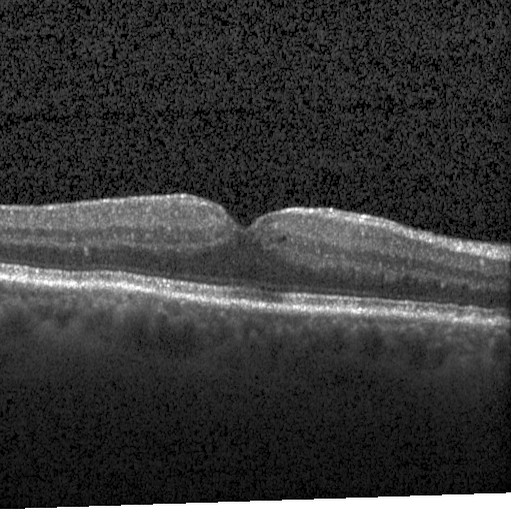

Impression: DME.